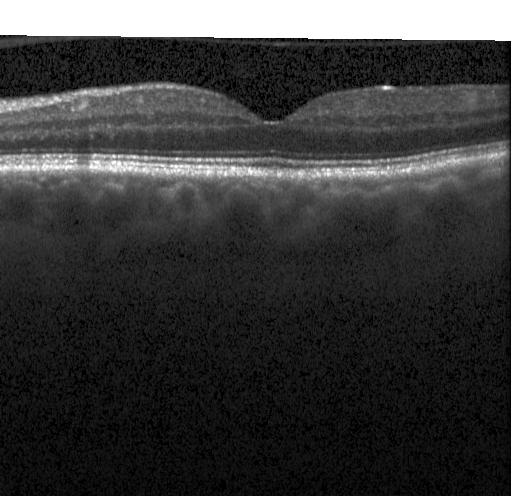

Optical coherence tomography scan; Heidelberg Spectralis OCT system; spectral-domain optical coherence tomography. Assessment: neither CNV, DME, nor drusen.